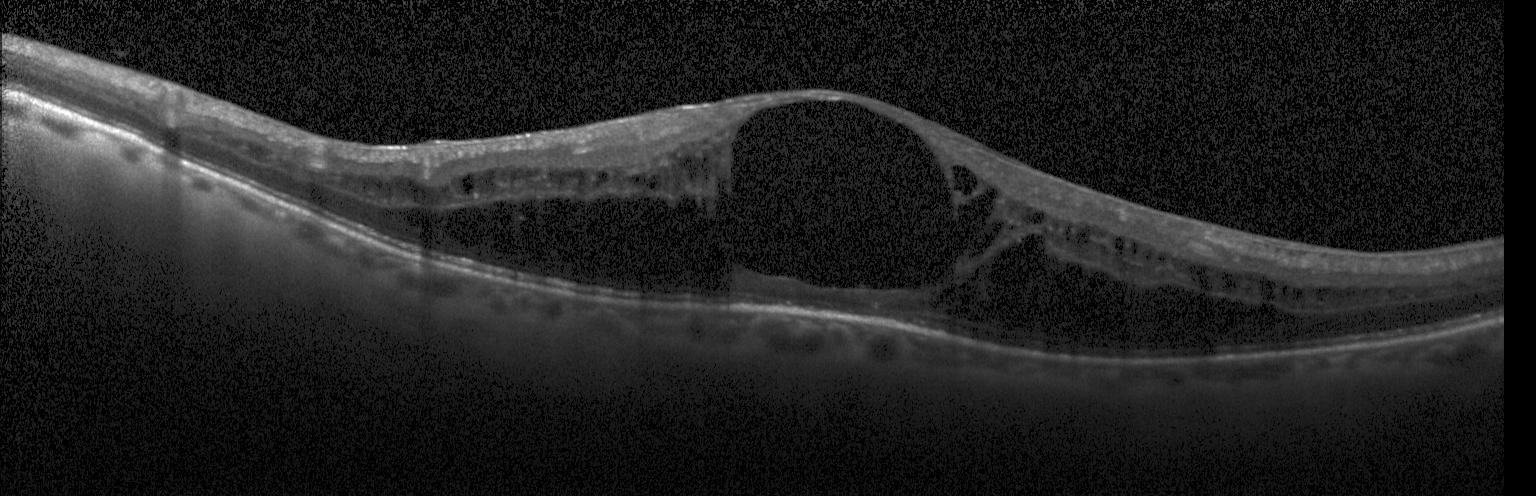

OCT B-scan — Impression: diabetic macular edema (DME).